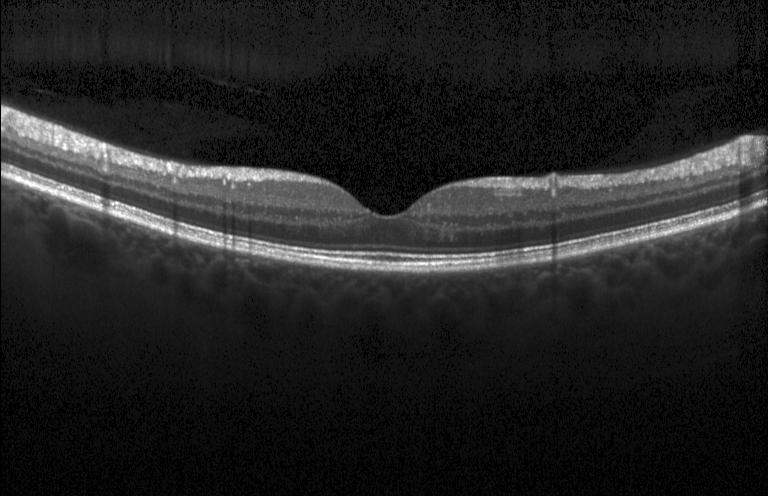

OCT line scan — Finding: no evidence of CNV, DME, or drusen.